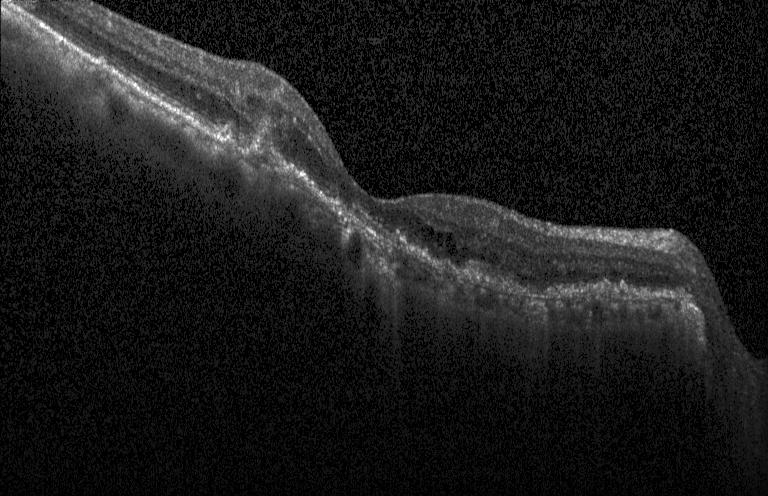 Diagnosis: a choroidal neovascular membrane.